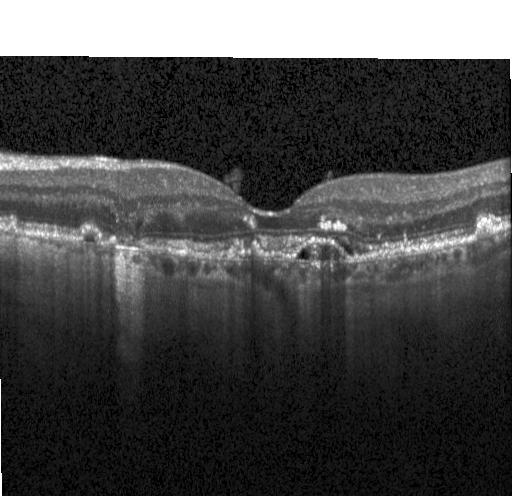

OCT line scan. SD-OCT. Finding: a choroidal neovascular membrane.